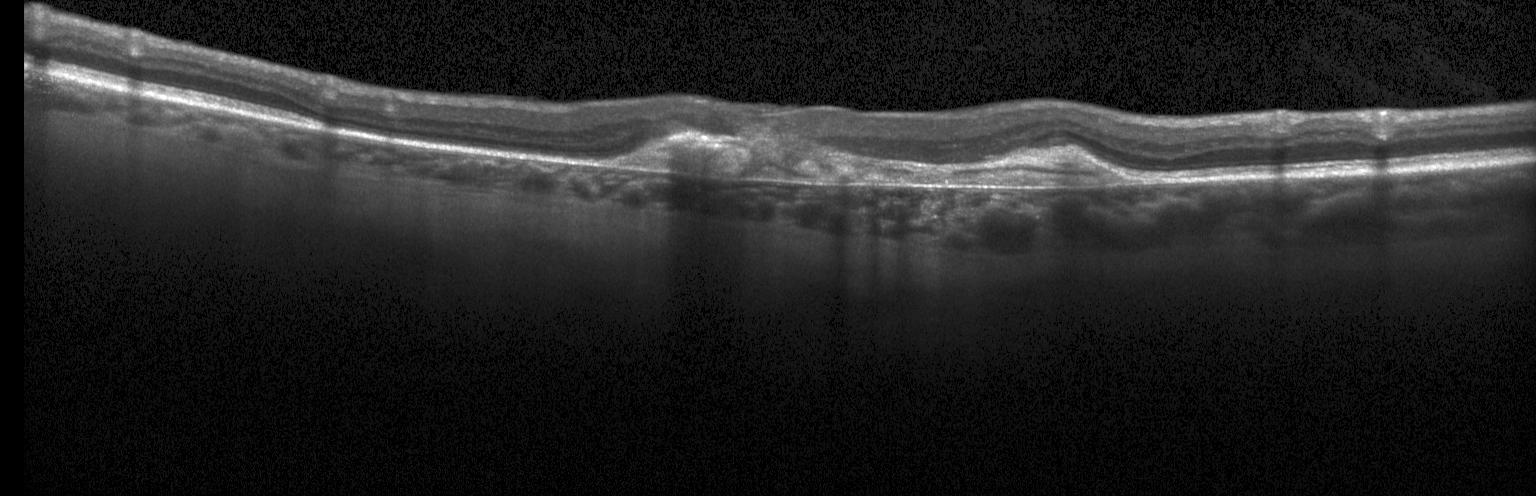
Centered on the fovea; retinal OCT B-scan; Heidelberg Spectralis
Impression: choroidal neovascularization.